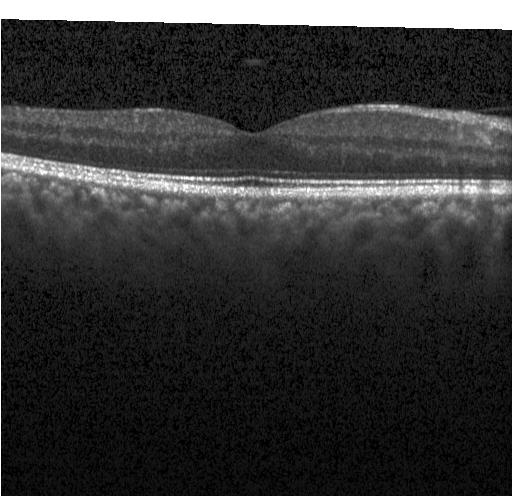

Optical coherence tomography B-scan.
Macular OCT: no evidence of choroidal neovascularization, diabetic macular edema, or drusen.